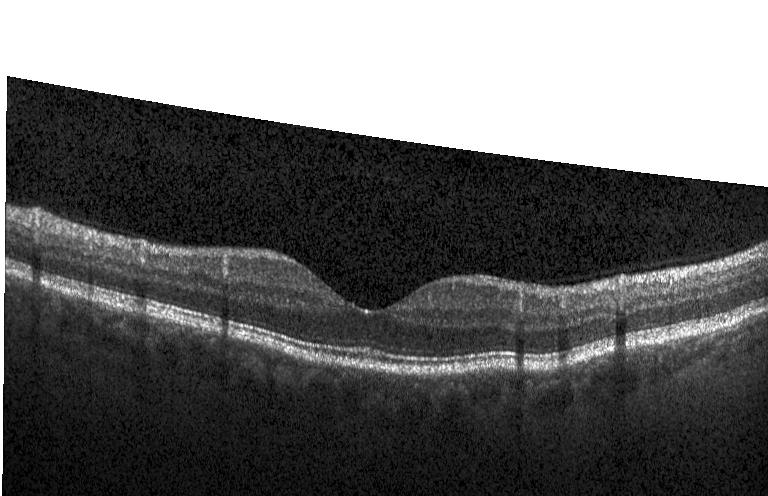
Assessment: neither choroidal neovascularization, diabetic macular edema, nor drusen.